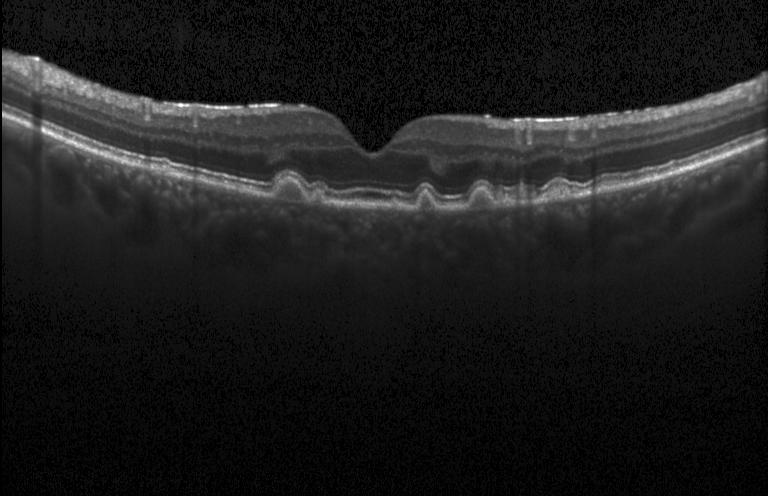
Diagnosis: multiple drusen.